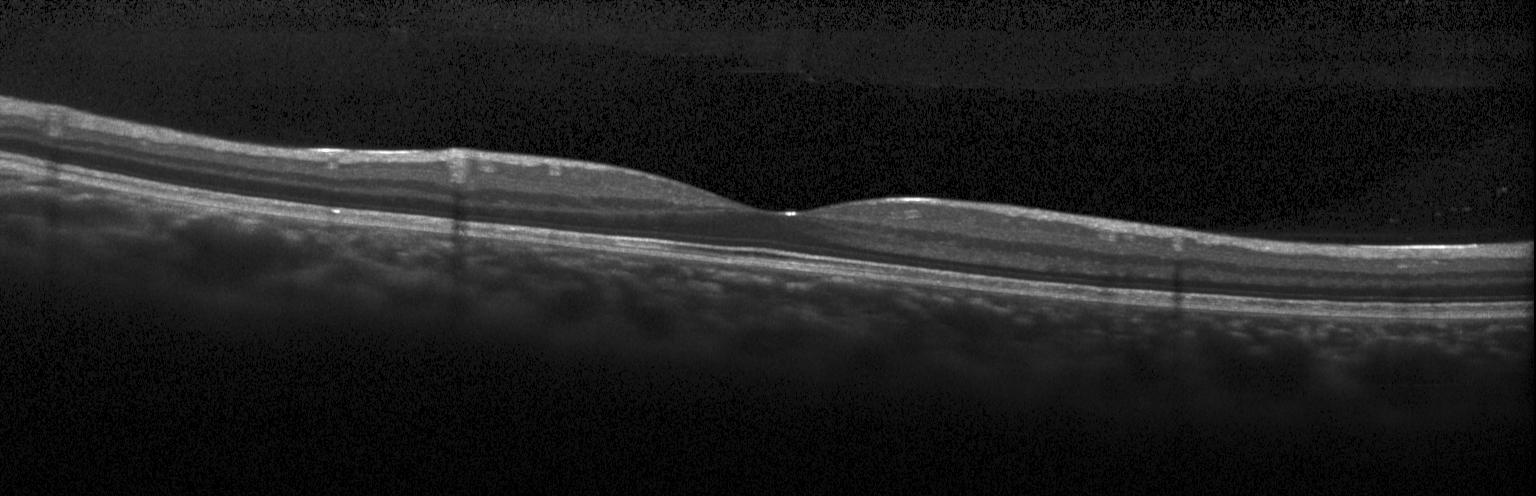

Retinal OCT cross-section. Heidelberg Spectralis OCT system. Macular scan. Impression: no choroidal neovascularization, diabetic macular edema, or drusen.